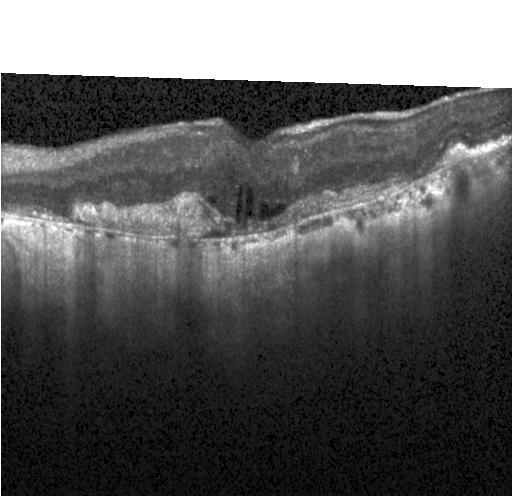
The scan shows choroidal neovascularization.